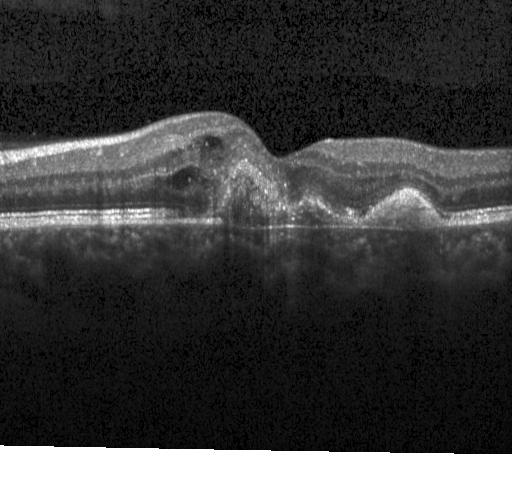 This B-scan demonstrates a choroidal neovascular membrane.